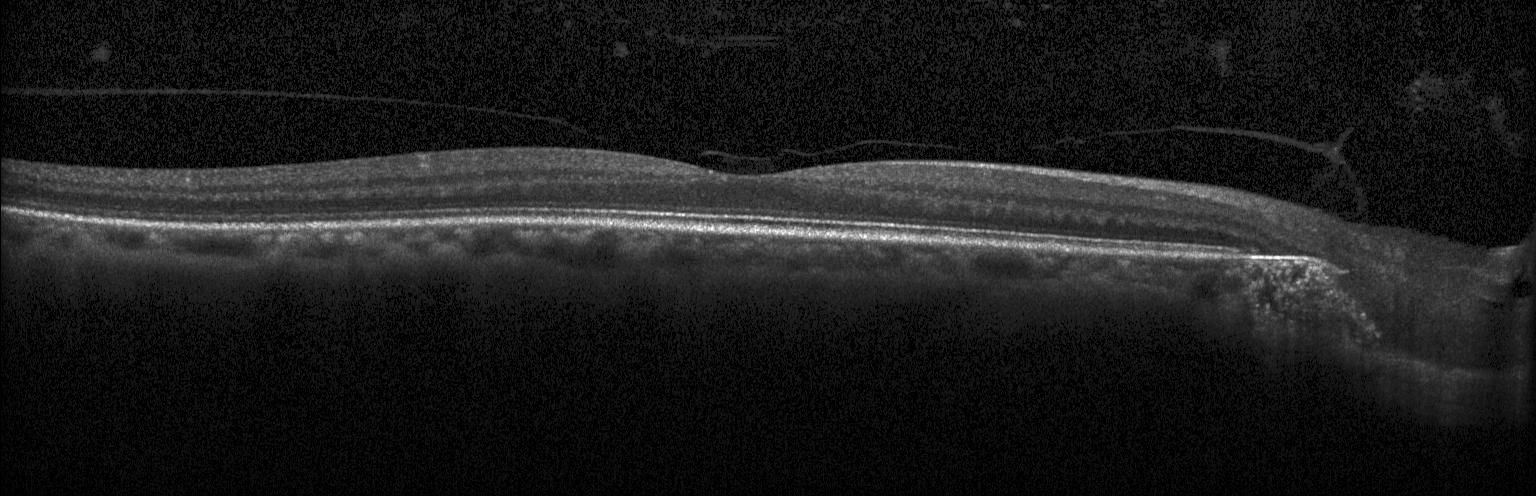 Impression: no choroidal neovascularization, diabetic macular edema, or drusen.